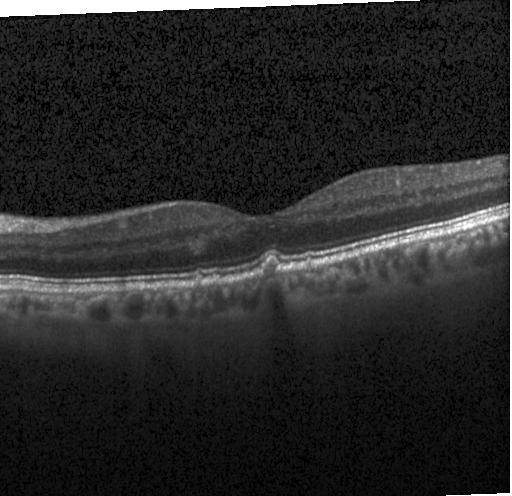

Diagnosis: drusen.